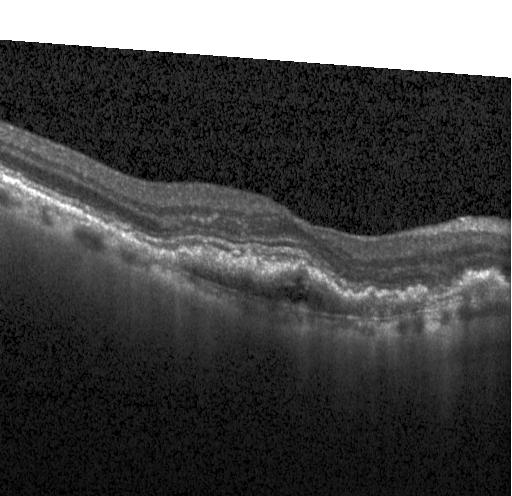
OCT finding: a choroidal neovascular membrane.